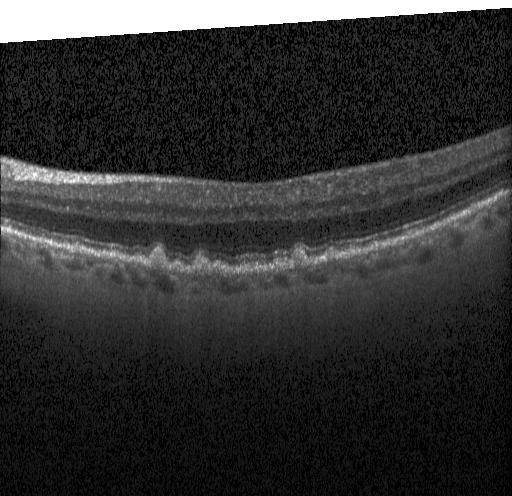

Macular scan. Spectral-domain optical coherence tomography. Optical coherence tomography B-scan.
Finding: multiple drusen.